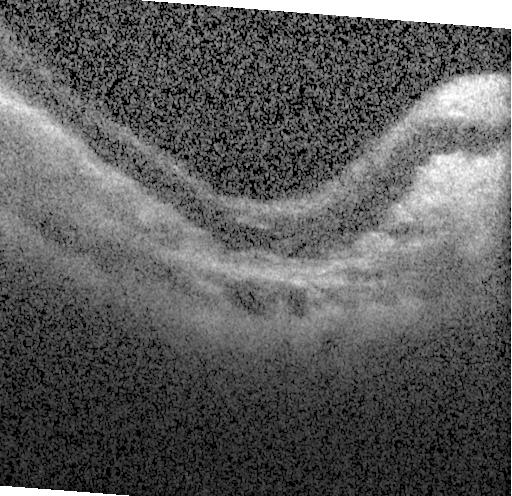

Horizontal scan through the fovea. OCT B-scan.
Macular OCT: a choroidal neovascular membrane.